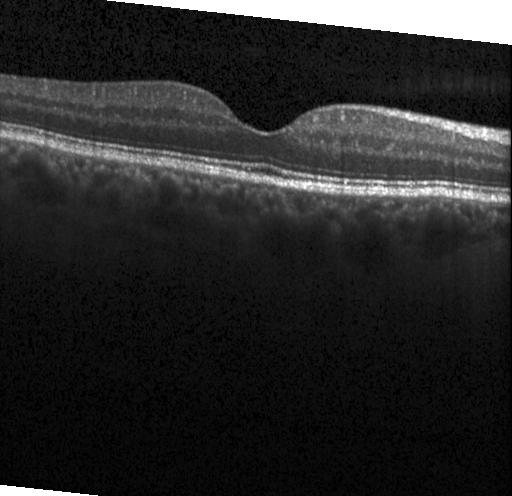

Acquired on a Heidelberg Spectralis, OCT line scan, horizontal scan through the fovea.
OCT finding: neither CNV, DME, nor drusen.